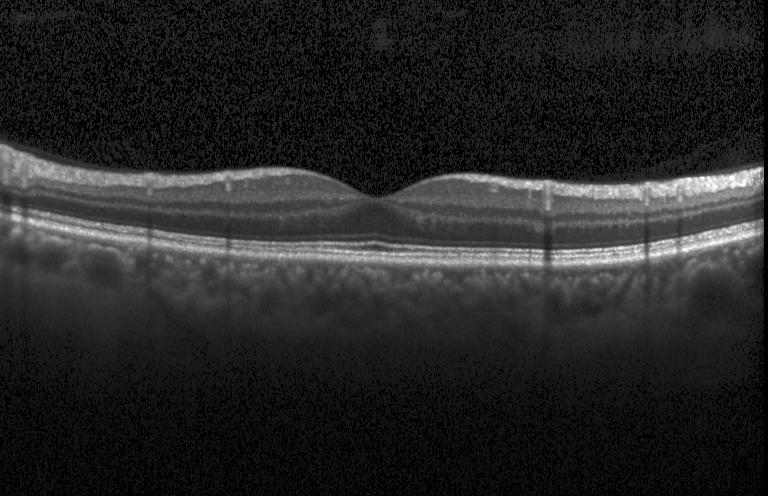

Optical coherence tomography B-scan. The scan shows no evidence of choroidal neovascularization, diabetic macular edema, or drusen.